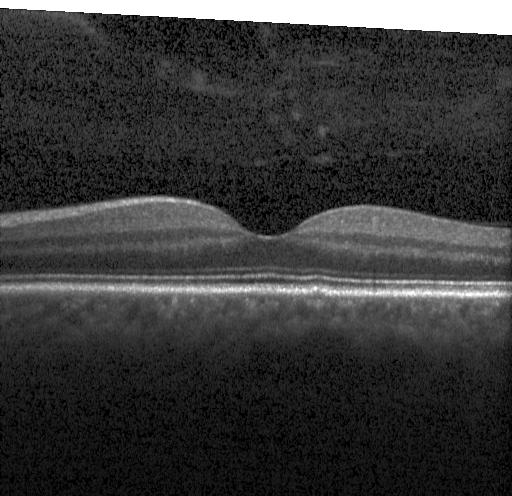
Retinal OCT cross-section — No CNV, DME, or drusen.